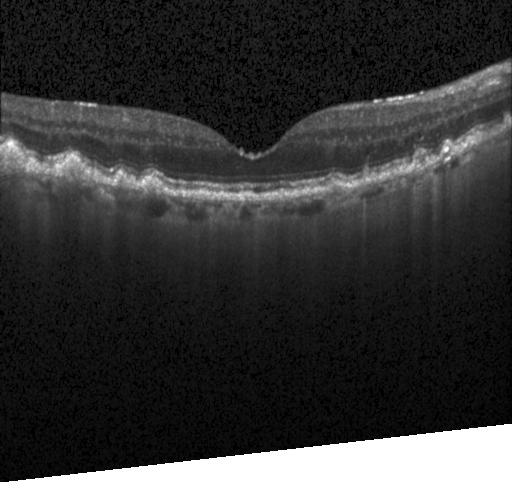

Macular OCT demonstrating drusen.